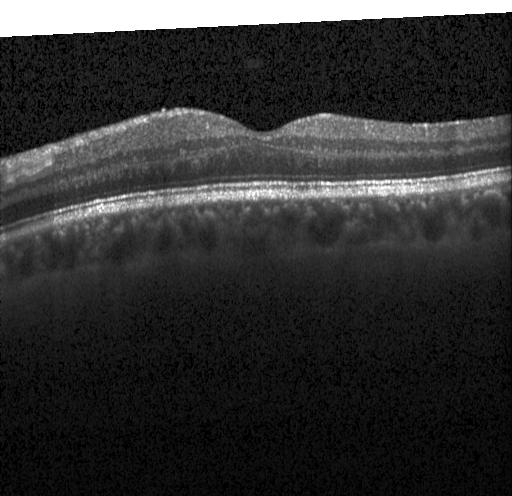

OCT B-scan. Impression: neither choroidal neovascularization, diabetic macular edema, nor drusen.